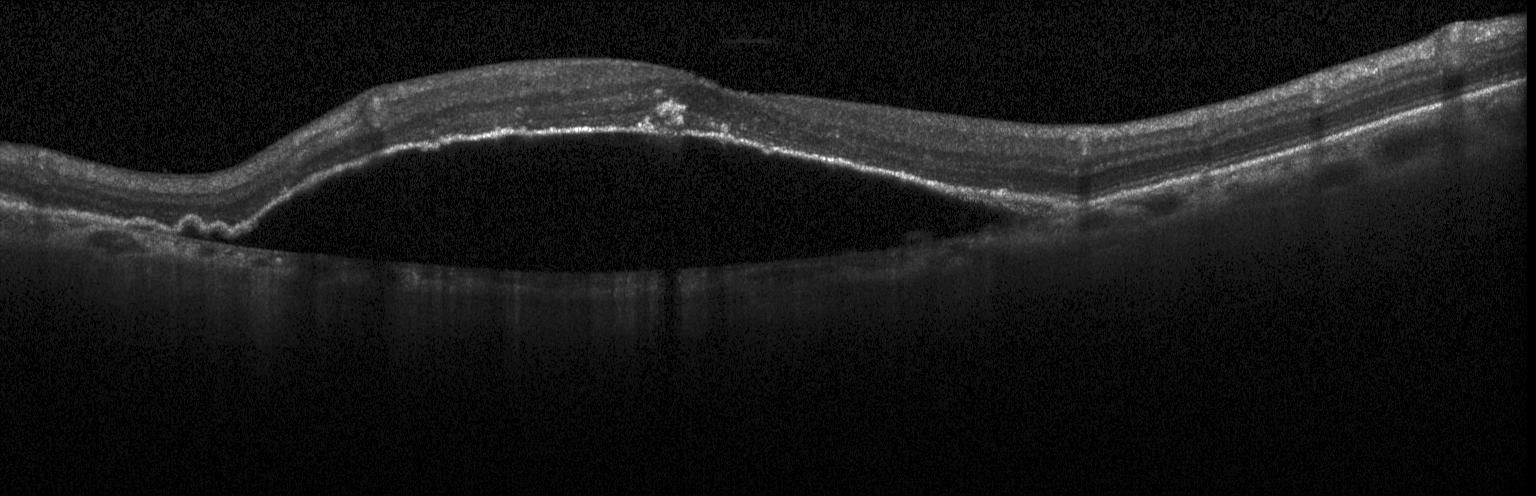 Retinal OCT cross-section. Acquired on a Heidelberg Spectralis — Dx: choroidal neovascularization (CNV).